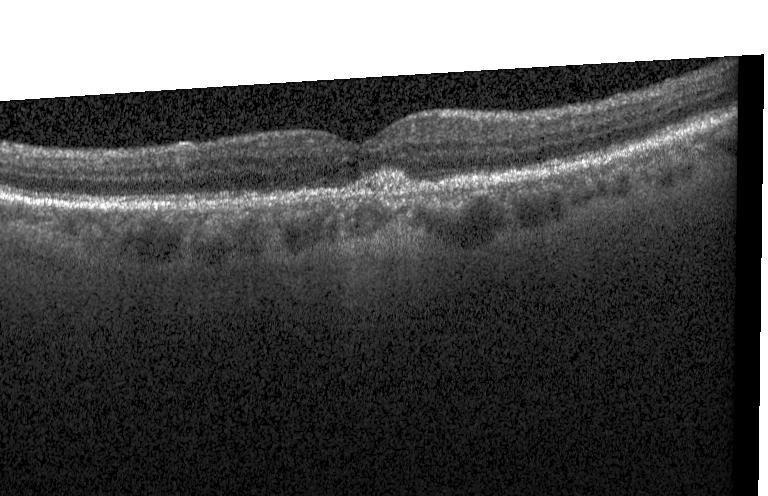

Spectral-domain optical coherence tomography; retinal OCT B-scan; centered on the fovea; acquired on a Heidelberg Spectralis — The scan shows choroidal neovascularization (CNV).